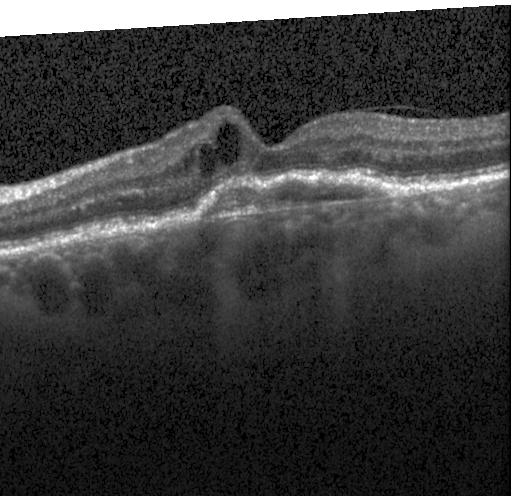 OCT finding: choroidal neovascularization.